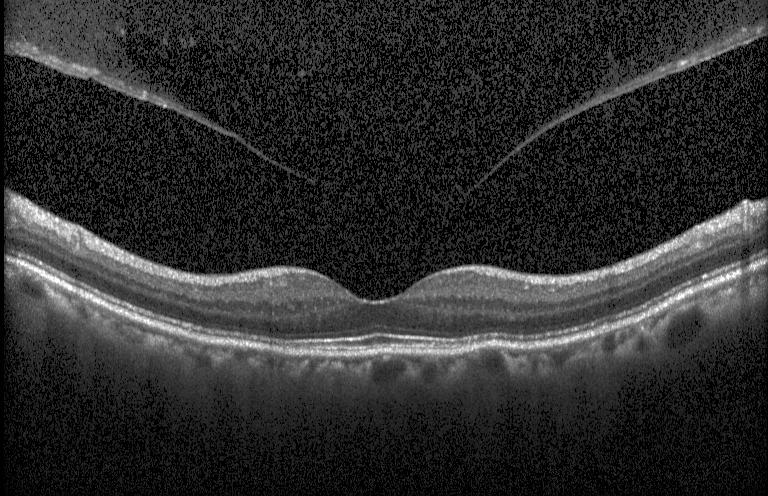
Retinal OCT cross-section. This B-scan demonstrates no evidence of CNV, DME, or drusen.